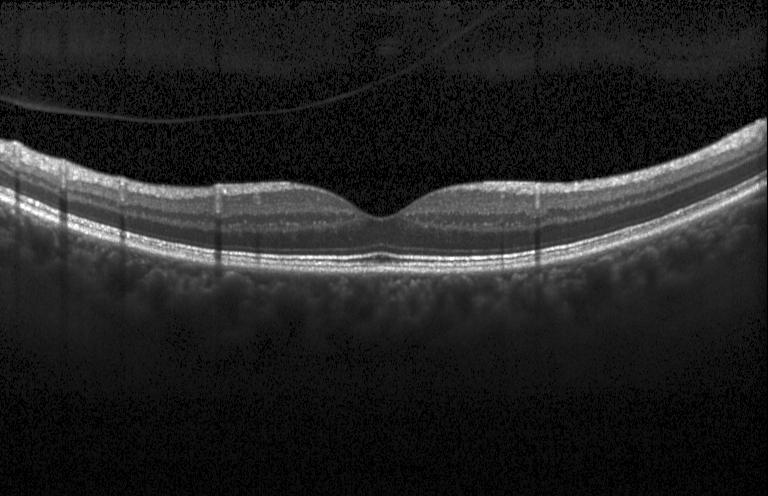 OCT finding: no evidence of choroidal neovascularization, diabetic macular edema, or drusen.